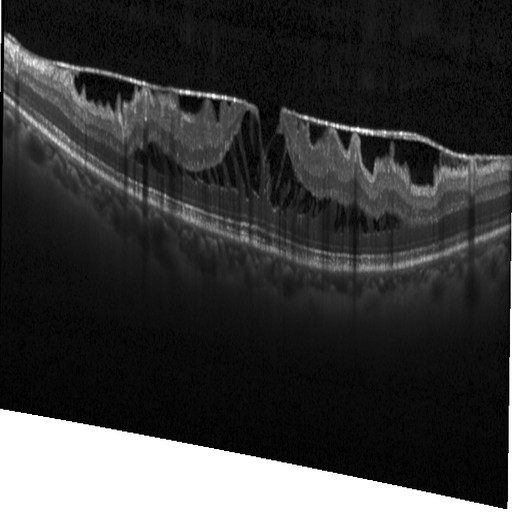 Diagnosis: diabetic macular edema.